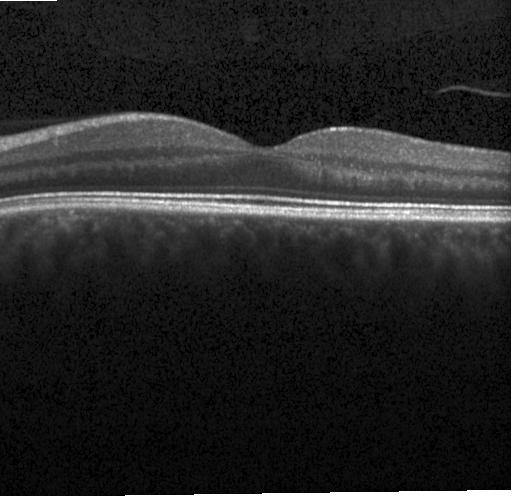
Heidelberg Spectralis · OCT B-scan · centered on the fovea — No CNV, DME, or drusen.